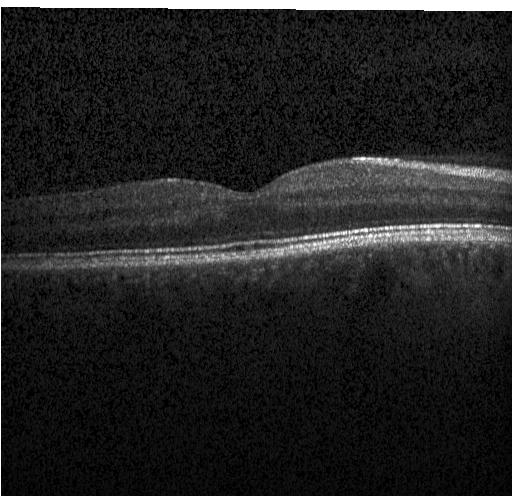 This B-scan demonstrates no choroidal neovascularization, no diabetic macular edema, and no drusen.